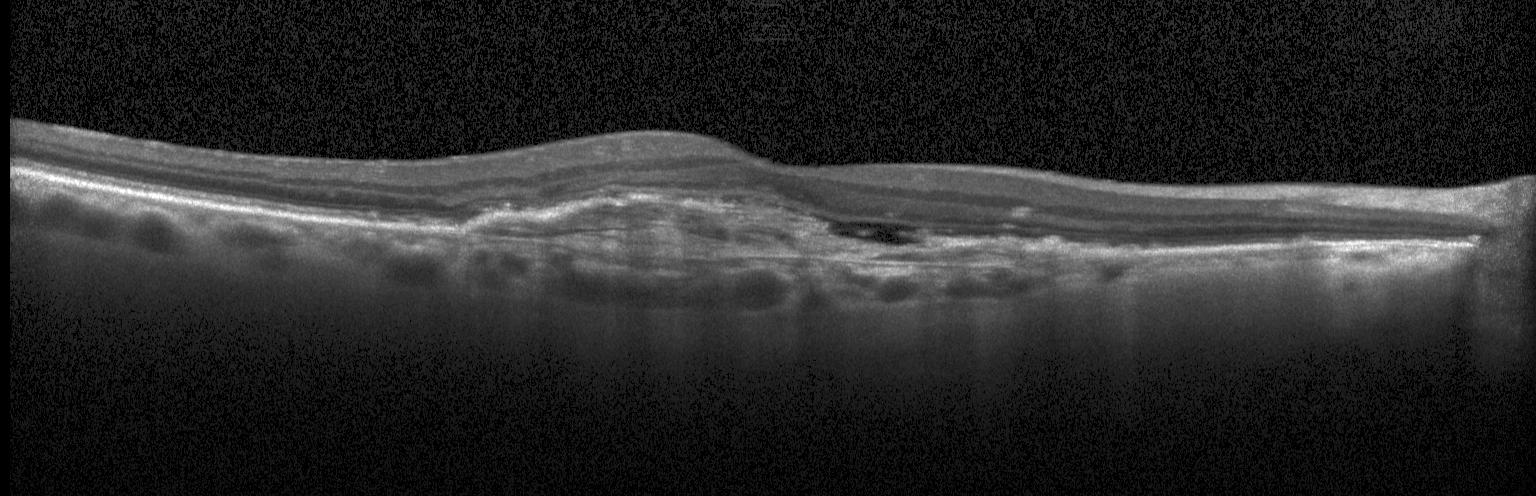 SD-OCT; retinal OCT B-scan; horizontal scan through the fovea.
Finding: choroidal neovascularization.